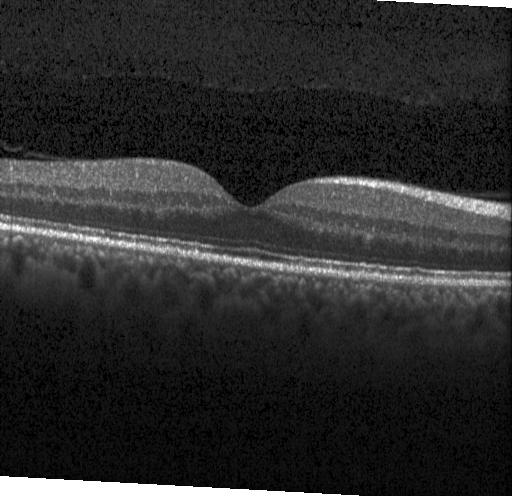
SD-OCT. Instrument: Heidelberg Spectralis. Centered on the fovea. Optical coherence tomography B-scan. Assessment: no choroidal neovascularization, no diabetic macular edema, and no drusen.